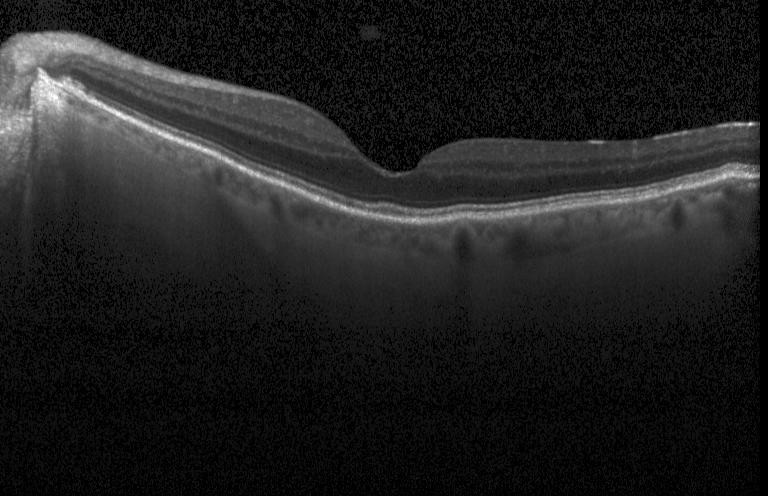
Assessment: no evidence of choroidal neovascularization, diabetic macular edema, or drusen.